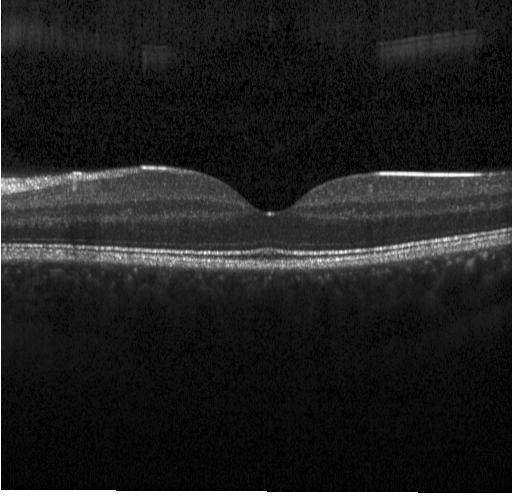

Retinal OCT B-scan; fovea-centered — Diagnosis: neither choroidal neovascularization, diabetic macular edema, nor drusen.